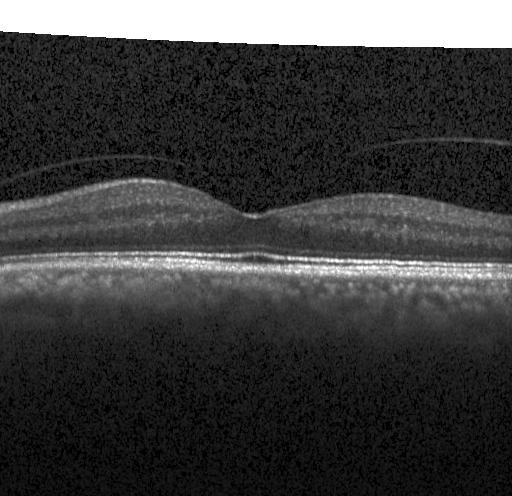 Diagnosis: no choroidal neovascularization, no diabetic macular edema, and no drusen.